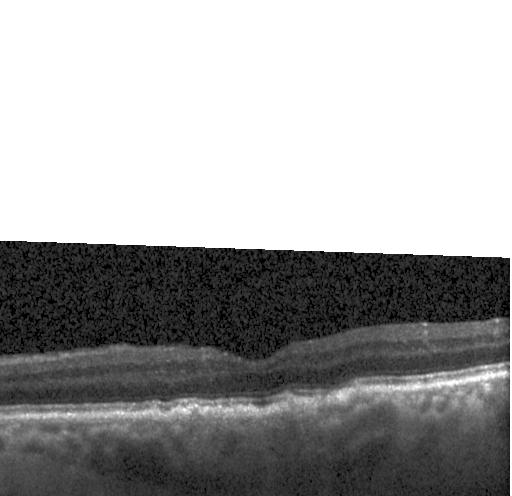

Horizontal scan through the fovea · SD-OCT · acquired on a Heidelberg Spectralis · optical coherence tomography scan. Diagnosis: sub-RPE drusenoid deposits.